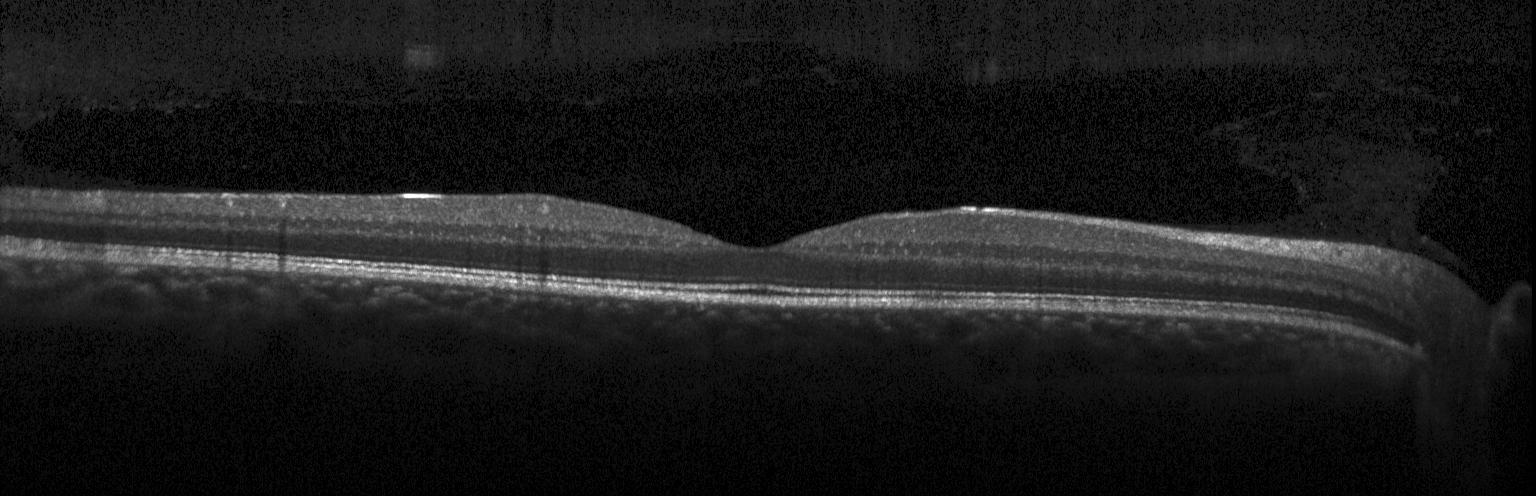 The scan shows no CNV, no DME, and no drusen.